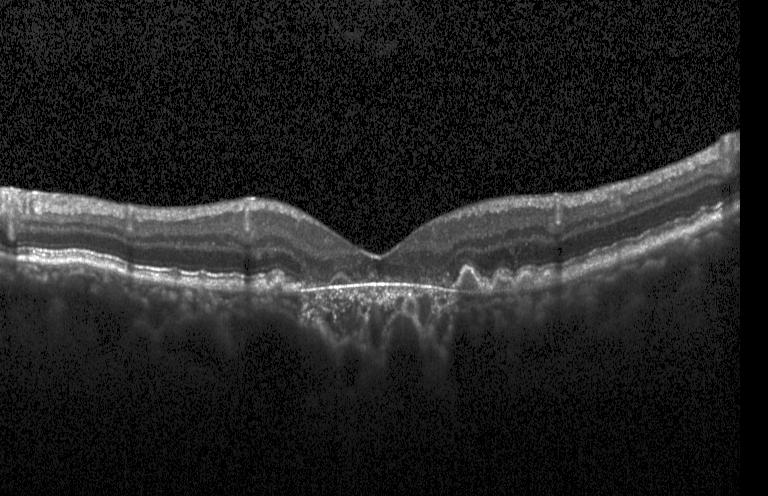

OCT B-scan. Dx: a choroidal neovascular membrane.